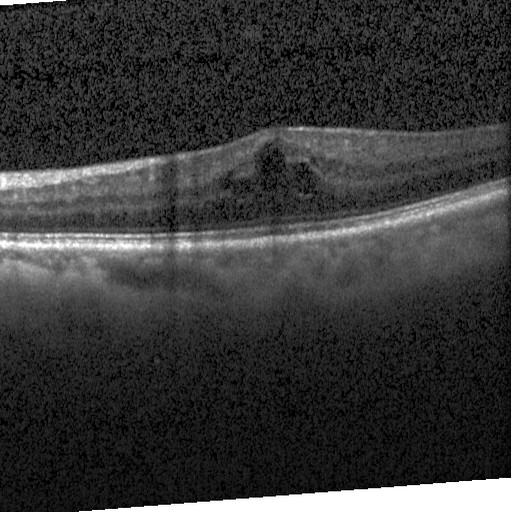
SD-OCT. Retinal OCT cross-section. Acquired on a Heidelberg Spectralis. Centered on the fovea
Diagnosis: DME.